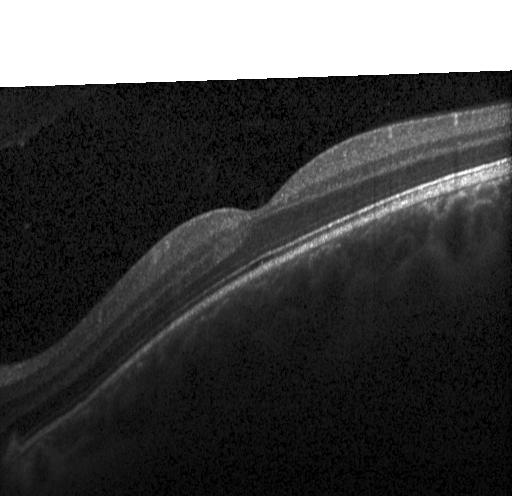
The scan shows neither choroidal neovascularization, diabetic macular edema, nor drusen.